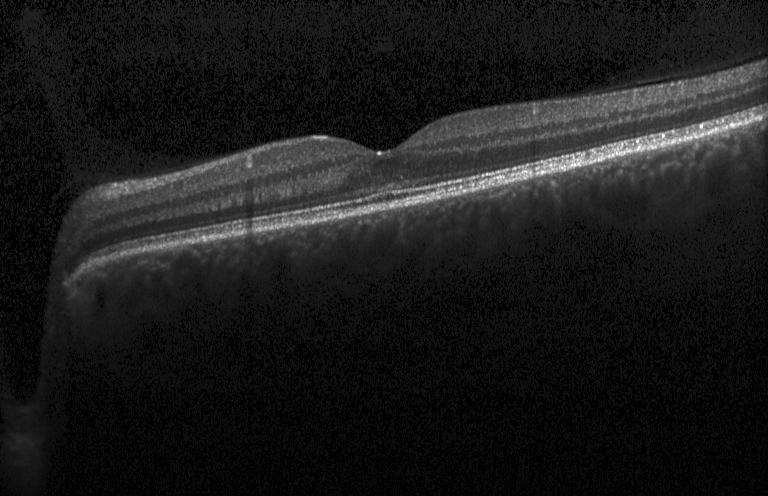

Optical coherence tomography B-scan; Heidelberg Spectralis — Assessment: no choroidal neovascularization, no diabetic macular edema, and no drusen.